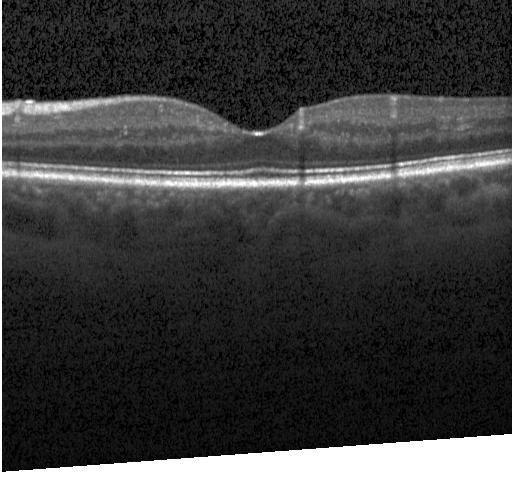

Retinal OCT B-scan, acquired on a Heidelberg Spectralis, spectral-domain OCT, through the macula. OCT finding: no choroidal neovascularization, no diabetic macular edema, and no drusen.